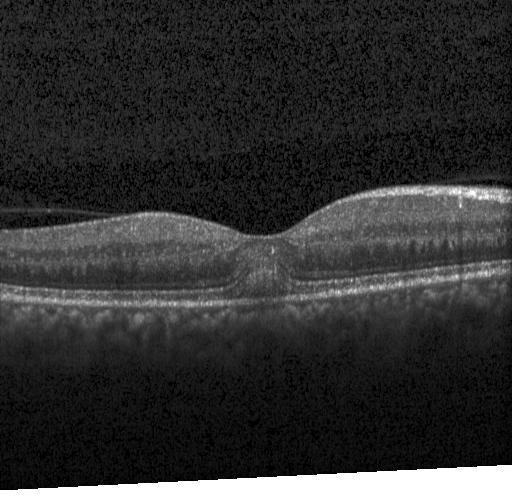

Horizontal scan through the fovea, spectral-domain optical coherence tomography, Heidelberg Spectralis OCT system, optical coherence tomography B-scan. A choroidal neovascular membrane.